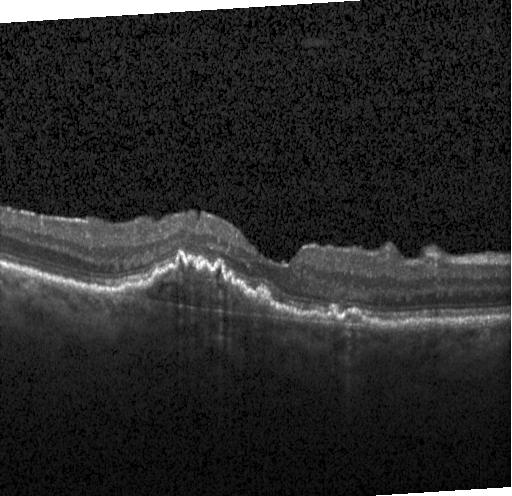 OCT B-scan showing choroidal neovascularization (CNV).